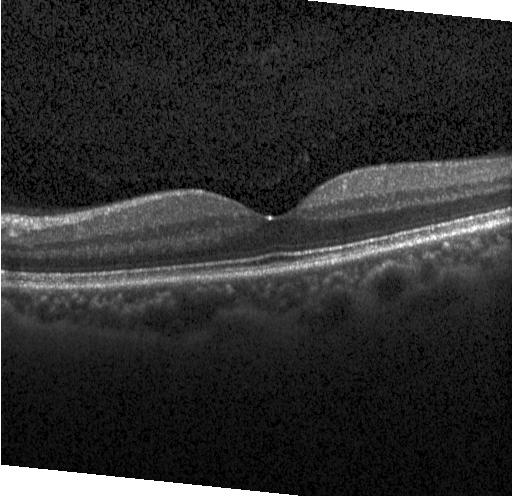 The scan shows no choroidal neovascularization, diabetic macular edema, or drusen.